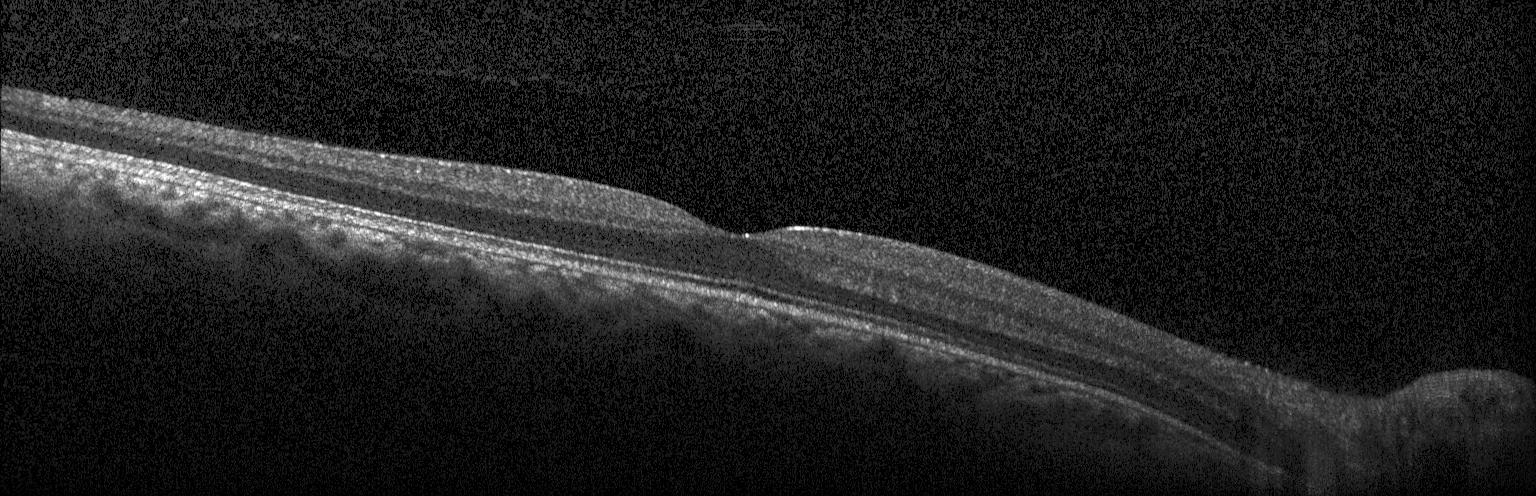
Optical coherence tomography scan, Heidelberg Spectralis. Assessment: no evidence of choroidal neovascularization, diabetic macular edema, or drusen.